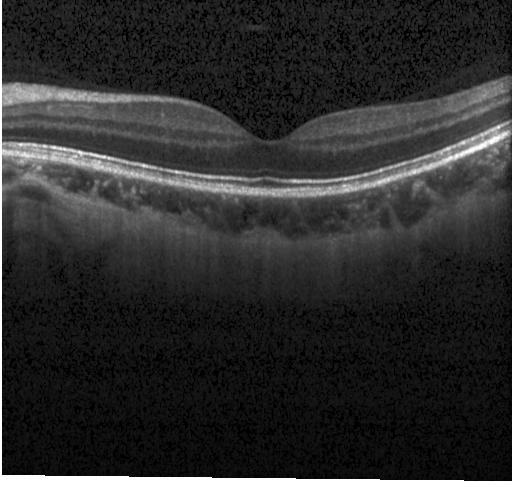
OCT finding: no CNV, no DME, and no drusen.